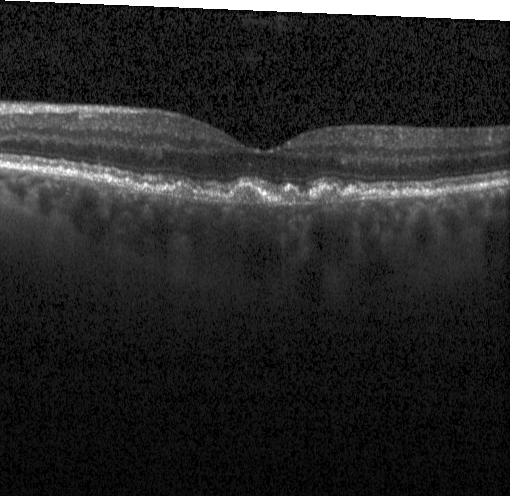

Centered on the fovea, optical coherence tomography scan
Finding: drusen.